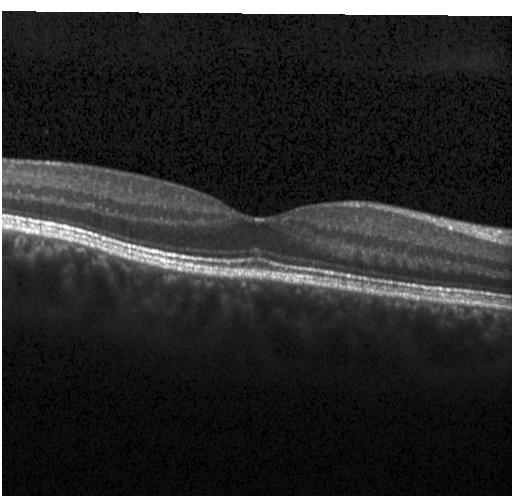
OCT line scan. Through the macula. The scan shows no CNV, DME, or drusen.